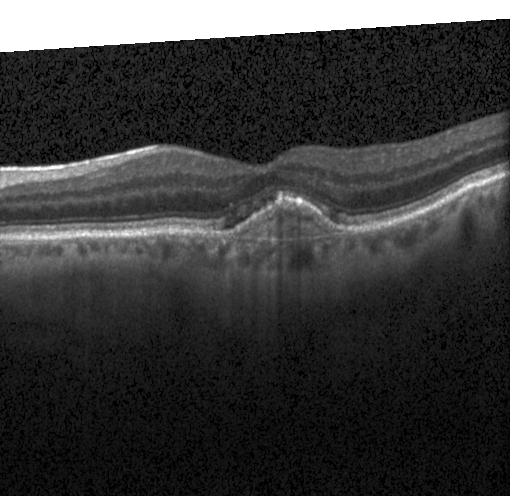 Assessment: CNV.